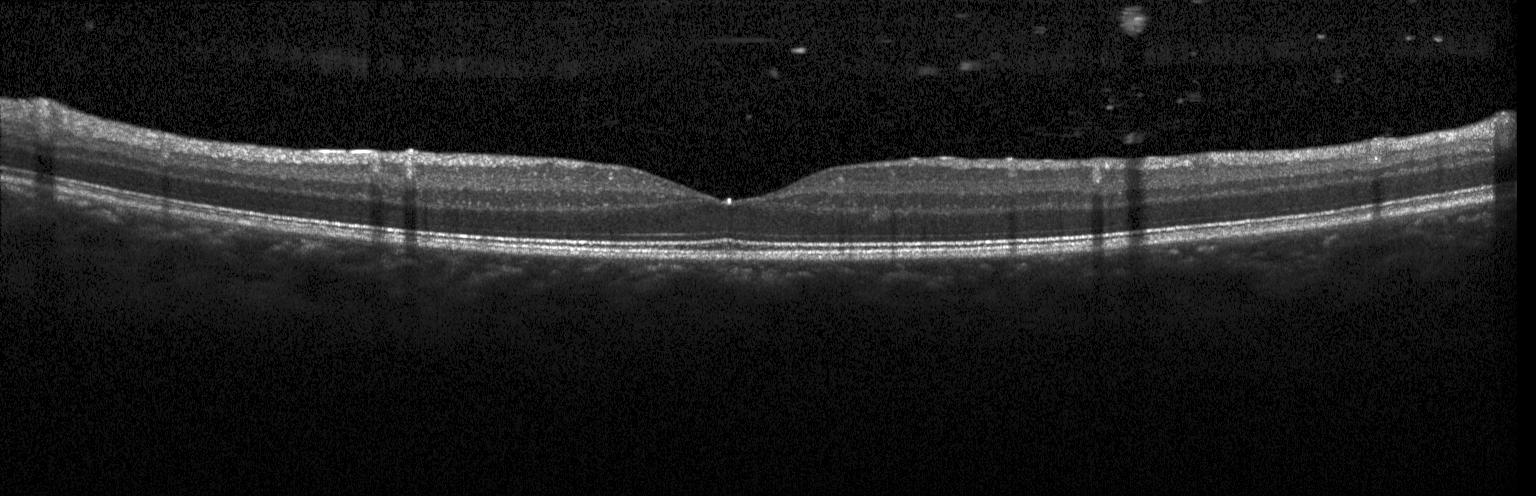 Spectral-domain optical coherence tomography; Heidelberg Spectralis OCT system; optical coherence tomography B-scan; macular scan. This B-scan demonstrates no evidence of choroidal neovascularization, diabetic macular edema, or drusen.